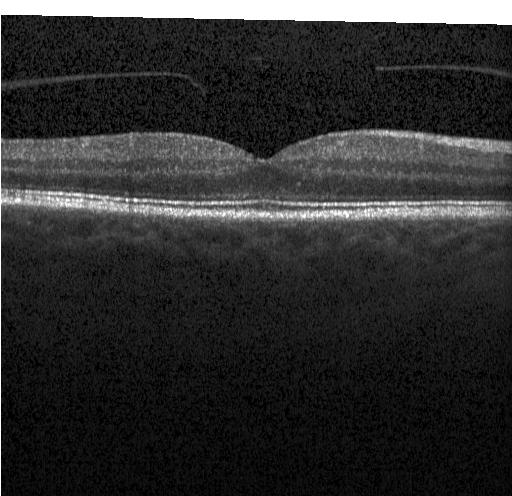
Acquired on a Heidelberg Spectralis, spectral-domain OCT, retinal OCT cross-section, macular scan
No evidence of choroidal neovascularization, diabetic macular edema, or drusen.